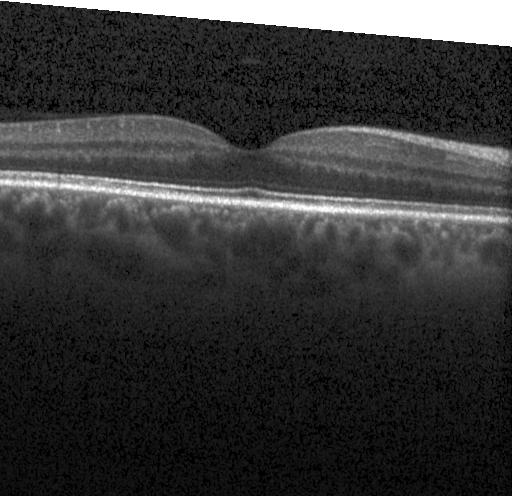
Retinal OCT B-scan
Assessment: no choroidal neovascularization, no diabetic macular edema, and no drusen.